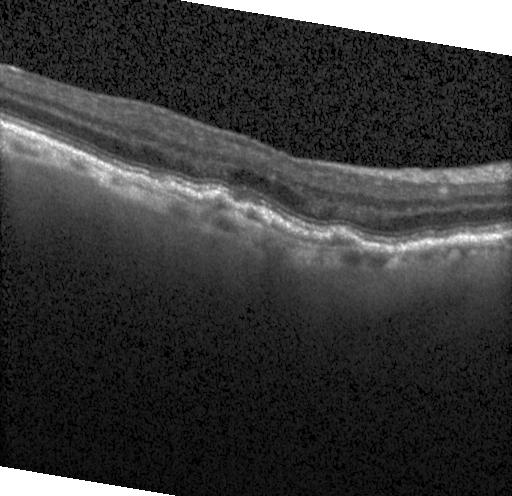 Acquired on a Heidelberg Spectralis. Spectral-domain OCT. Horizontal scan through the fovea. OCT line scan
A choroidal neovascular membrane.